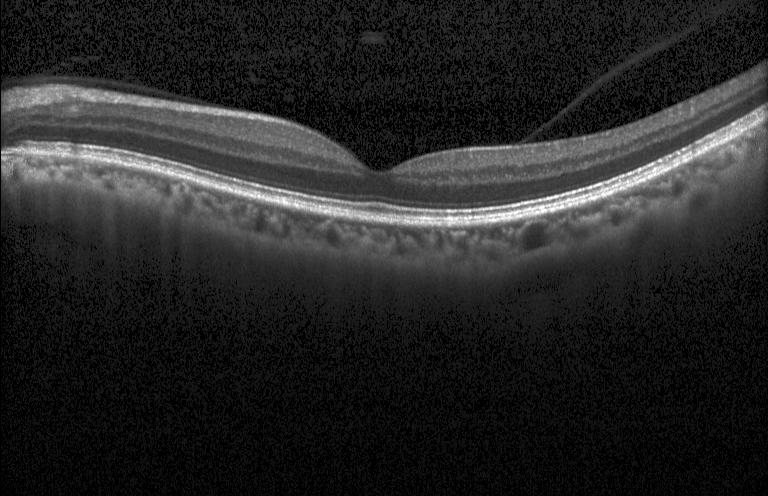 Macular scan · OCT line scan
No evidence of CNV, DME, or drusen.